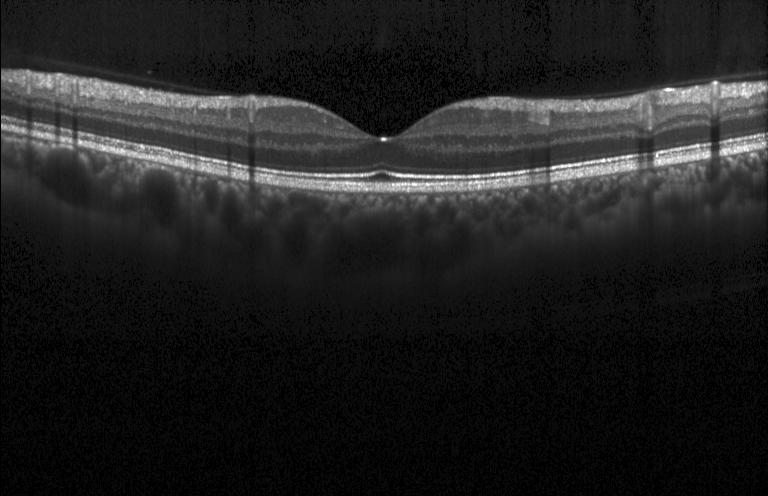
Retinal OCT cross-section; instrument: Heidelberg Spectralis; macular scan.
Finding: no evidence of choroidal neovascularization, diabetic macular edema, or drusen.